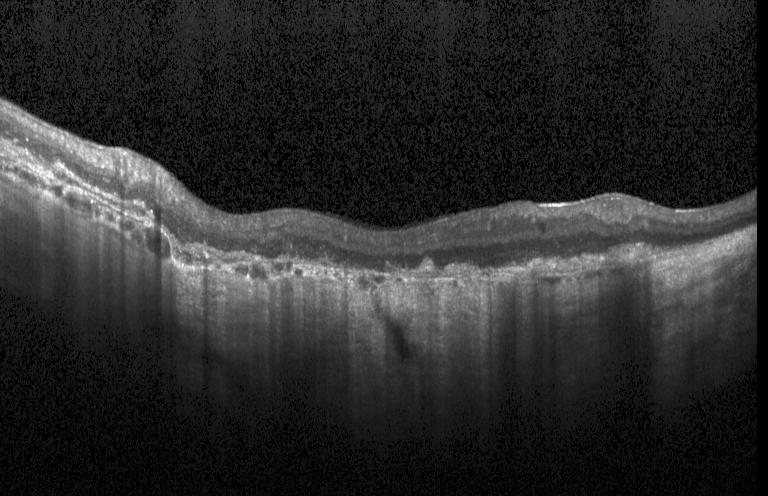
Assessment: a choroidal neovascular membrane.